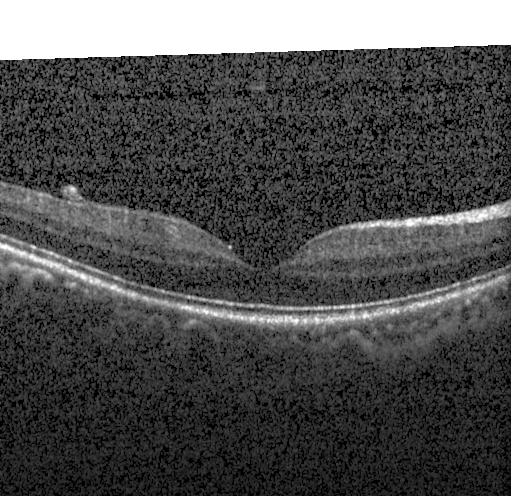
Retinal OCT cross-section; Heidelberg Spectralis OCT system; horizontal scan through the fovea; spectral-domain OCT.
No evidence of choroidal neovascularization, diabetic macular edema, or drusen.